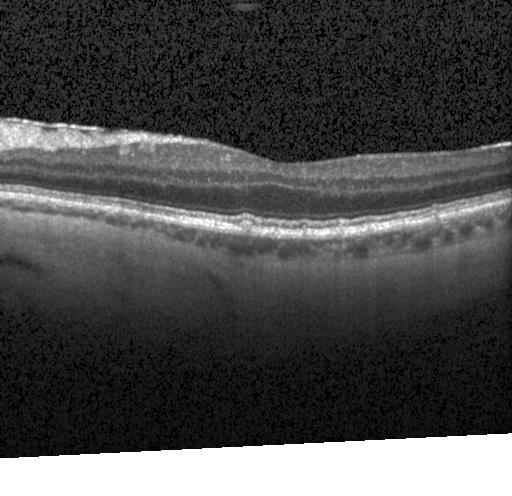 OCT line scan, Heidelberg Spectralis, spectral-domain optical coherence tomography, macular scan
Dx: multiple drusen.